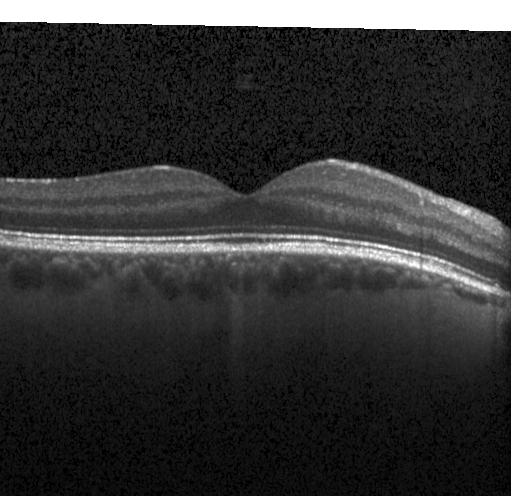

Instrument: Heidelberg Spectralis. OCT line scan. Spectral-domain optical coherence tomography. Through the macula.
Finding: no choroidal neovascularization, diabetic macular edema, or drusen.